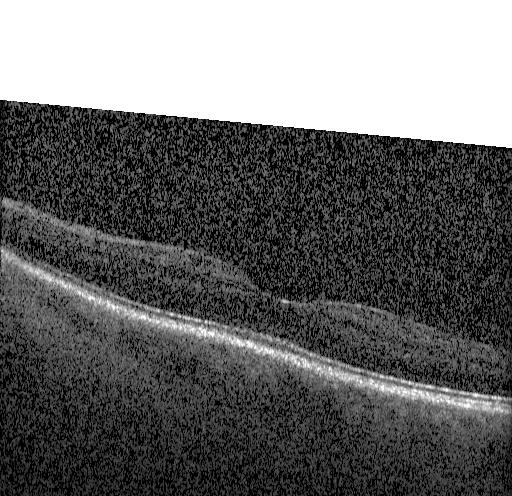 Impression: no choroidal neovascularization, no diabetic macular edema, and no drusen.